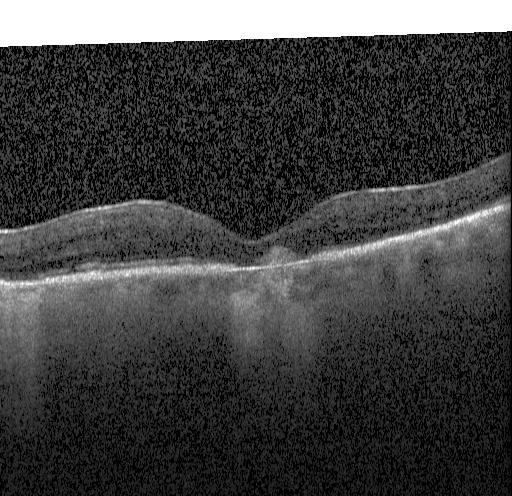 OCT finding: choroidal neovascularization (CNV).